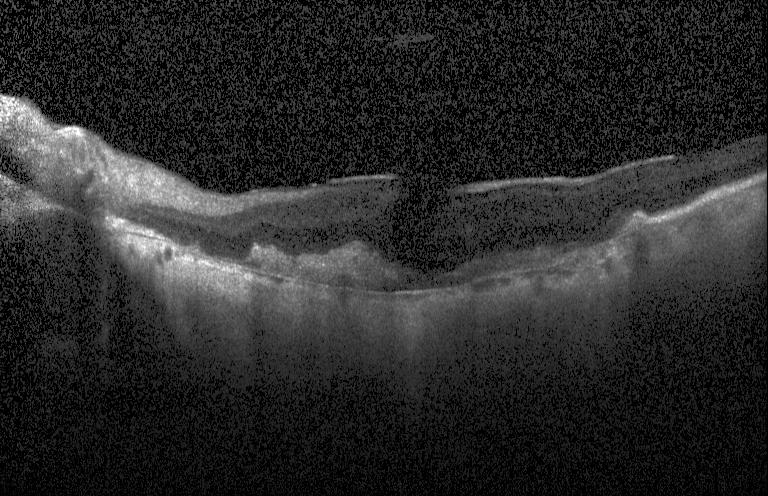
OCT B-scan showing a choroidal neovascular membrane.